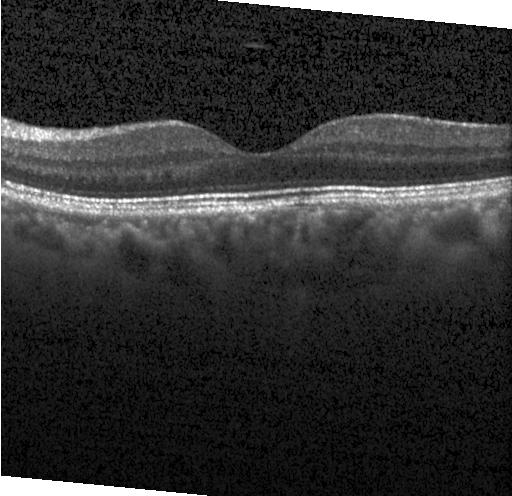 Optical coherence tomography scan. The scan shows no CNV, DME, or drusen.